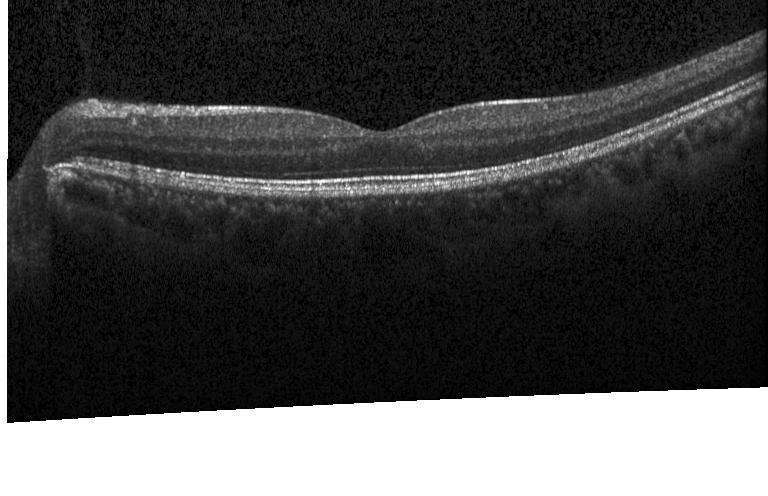

Optical coherence tomography B-scan; macular scan
The scan shows no choroidal neovascularization, no diabetic macular edema, and no drusen.